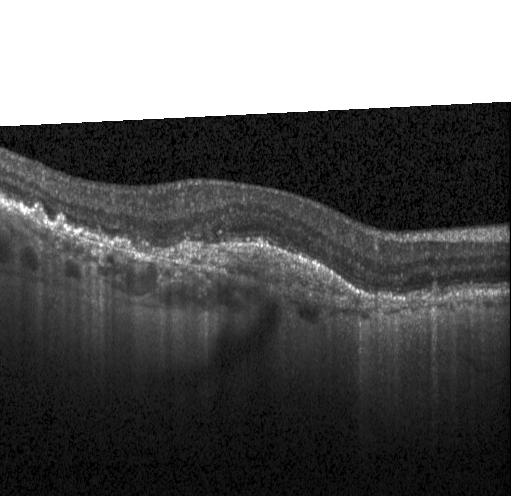 Acquired on a Heidelberg Spectralis · horizontal scan through the fovea · retinal OCT B-scan · spectral-domain optical coherence tomography.
Assessment: choroidal neovascularization.